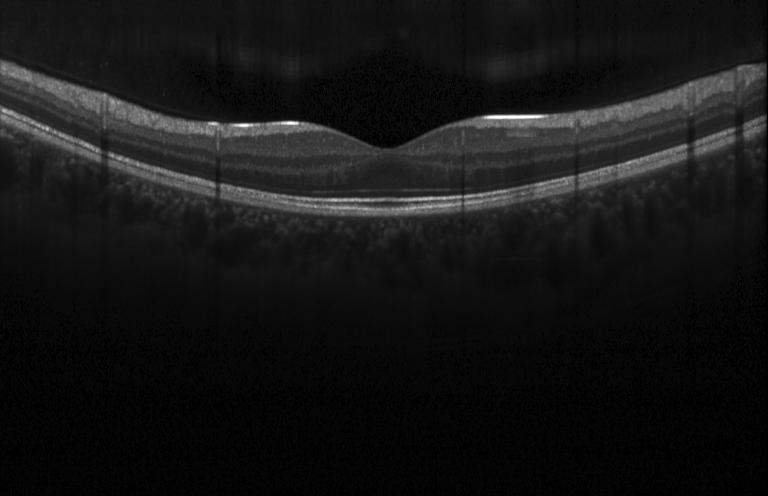
Instrument: Heidelberg Spectralis · retinal OCT cross-section
Neither choroidal neovascularization, diabetic macular edema, nor drusen.